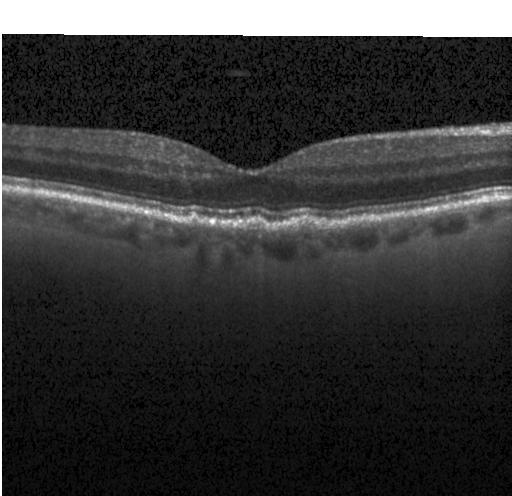

Macular OCT demonstrating multiple drusen.